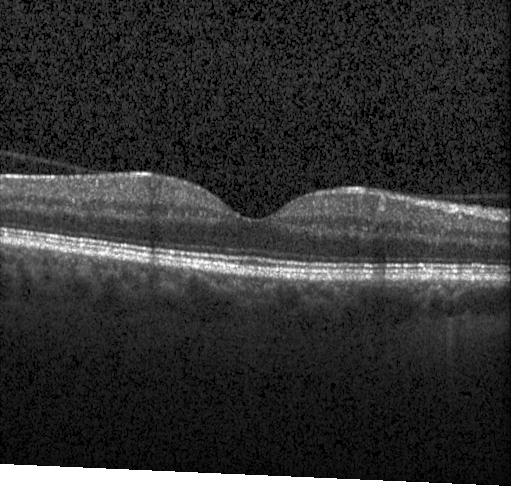

Dx: no choroidal neovascularization, no diabetic macular edema, and no drusen.